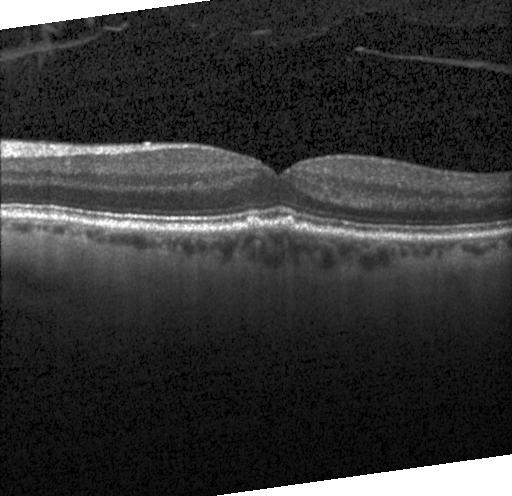

Macular OCT demonstrating sub-RPE drusenoid deposits.